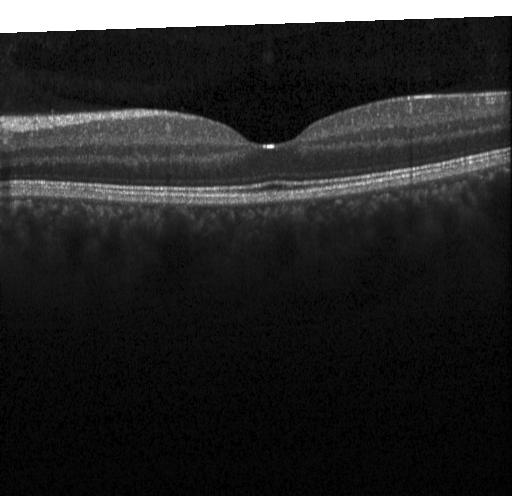 OCT line scan. This B-scan demonstrates neither choroidal neovascularization, diabetic macular edema, nor drusen.